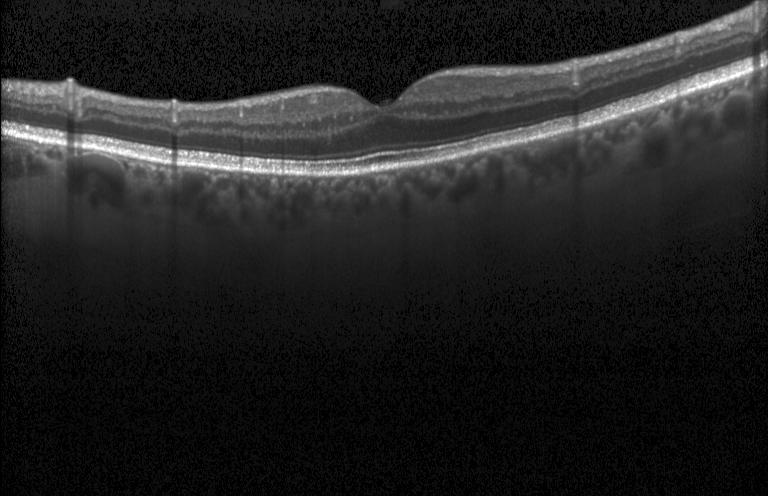 SD-OCT. Optical coherence tomography scan — OCT finding: no evidence of choroidal neovascularization, diabetic macular edema, or drusen.